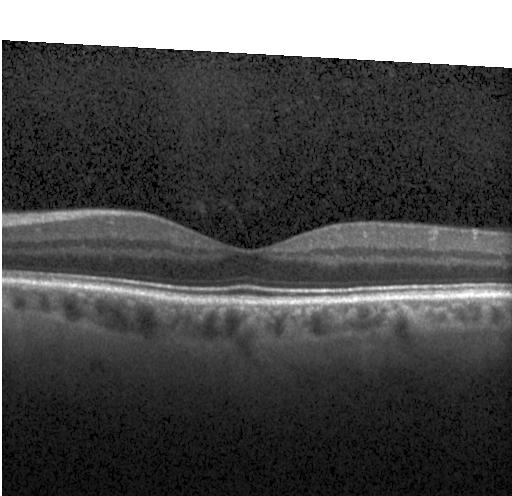
OCT line scan — Diagnosis: no choroidal neovascularization, diabetic macular edema, or drusen.